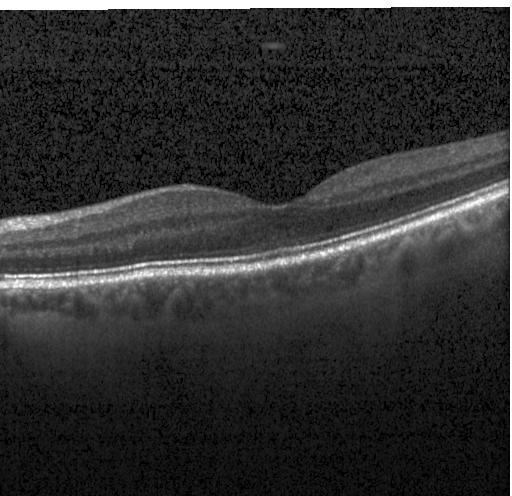

OCT B-scan · through the macula. The scan shows no evidence of choroidal neovascularization, diabetic macular edema, or drusen.